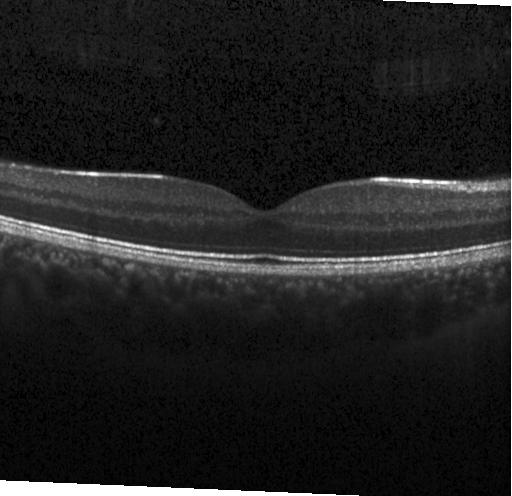

Macular OCT: no choroidal neovascularization, no diabetic macular edema, and no drusen.